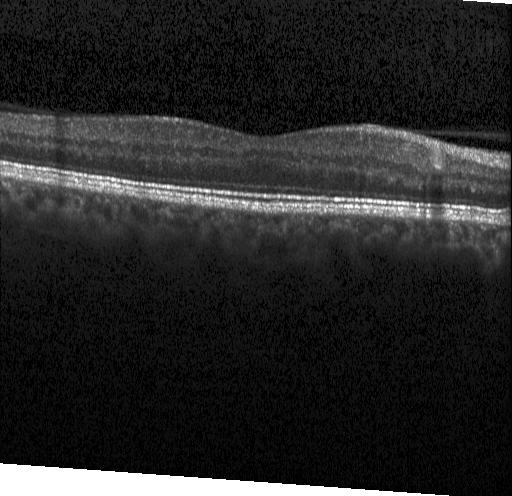
OCT scan showing no CNV, DME, or drusen.